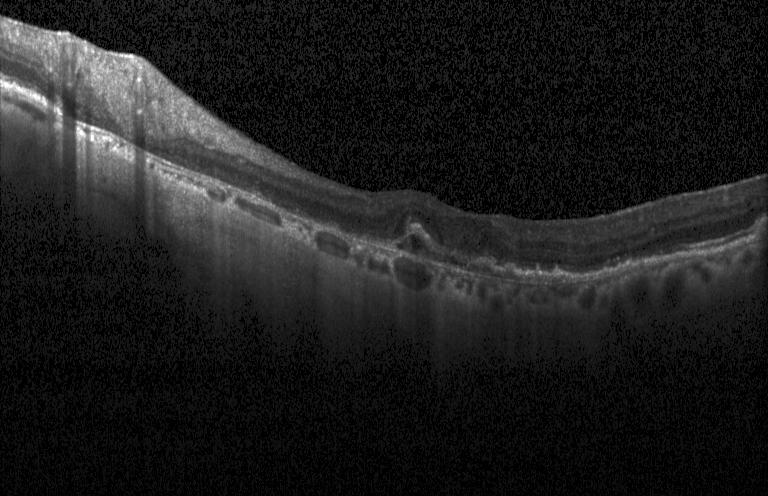
OCT line scan.
Diagnosis: a choroidal neovascular membrane.